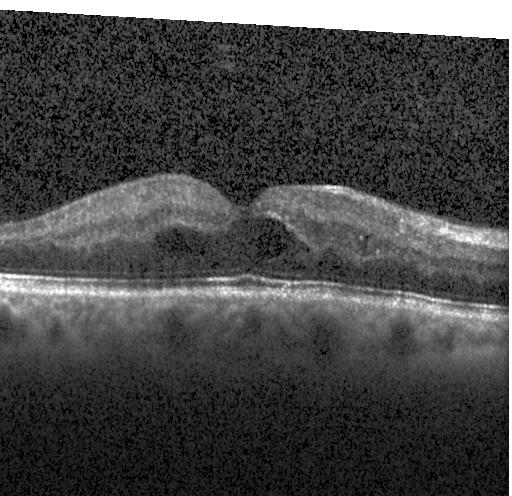 Macular OCT: diabetic macular edema.